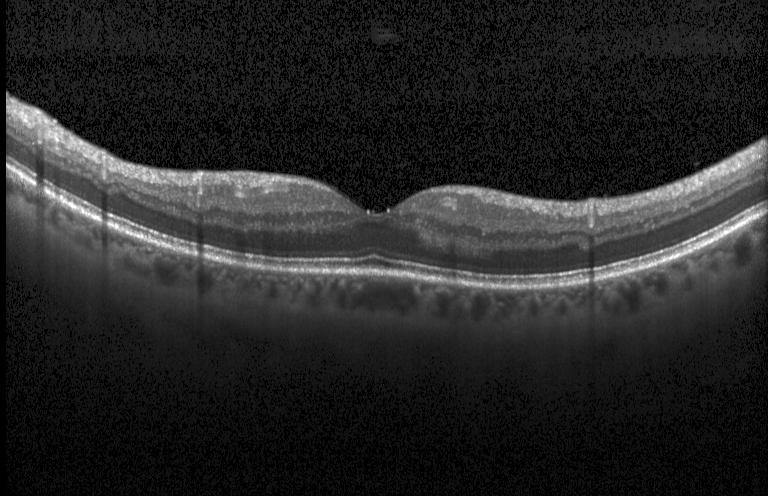

Finding: no choroidal neovascularization, no diabetic macular edema, and no drusen.